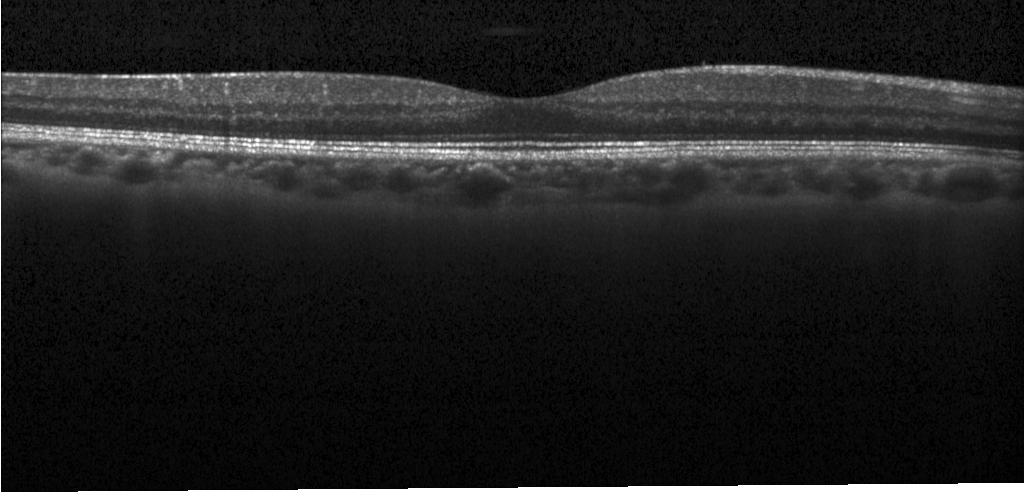
No choroidal neovascularization, no diabetic macular edema, and no drusen.